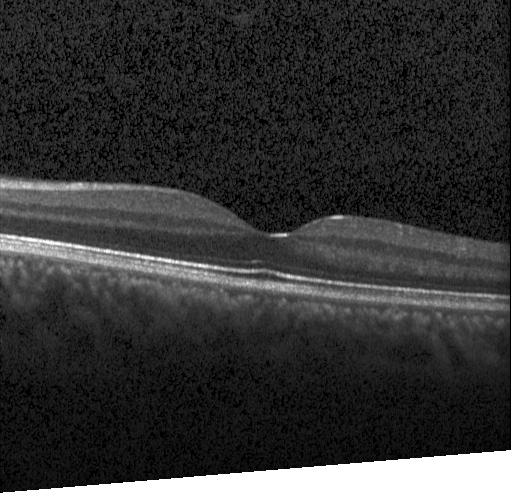 Through the macula, retinal OCT cross-section, acquired on a Heidelberg Spectralis. Dx: no choroidal neovascularization, diabetic macular edema, or drusen.